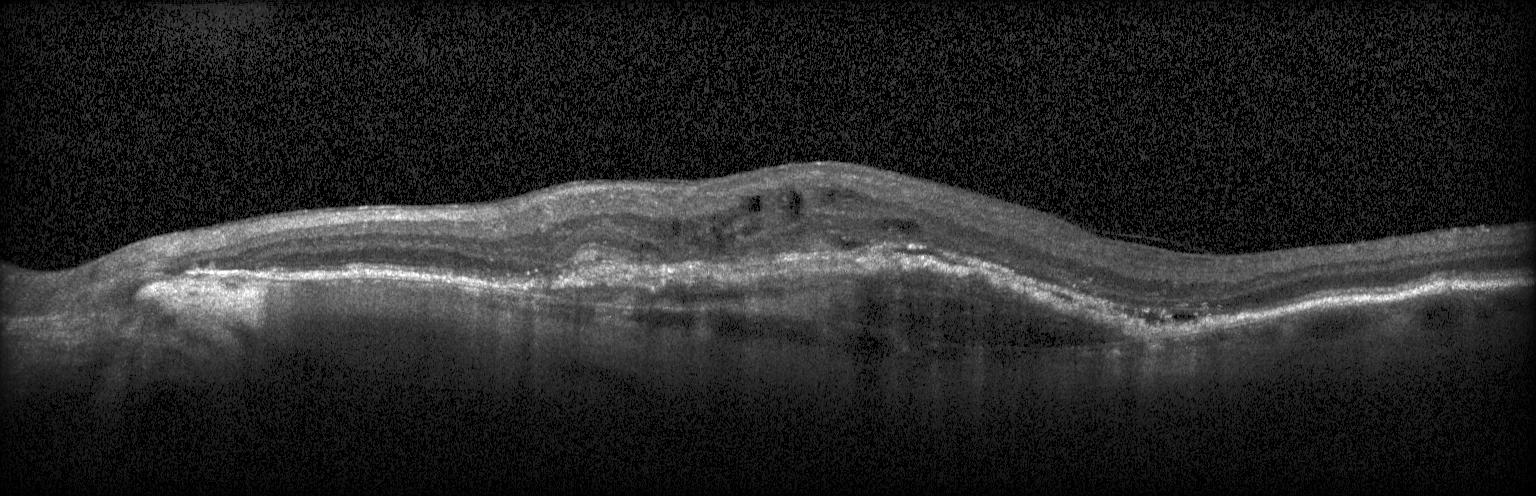
This B-scan demonstrates choroidal neovascularization (CNV).